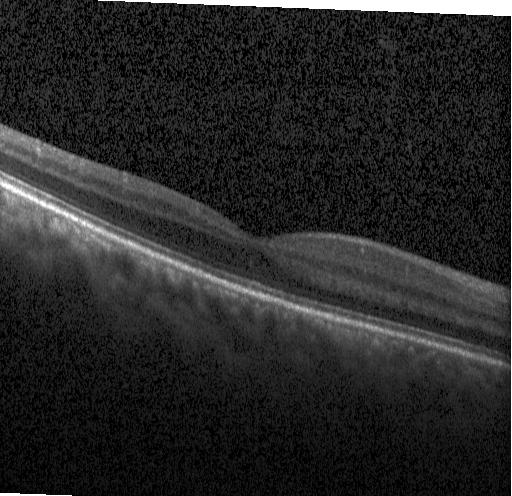

Spectral-domain OCT. Optical coherence tomography B-scan. Macular scan. Instrument: Heidelberg Spectralis.
Finding: neither choroidal neovascularization, diabetic macular edema, nor drusen.